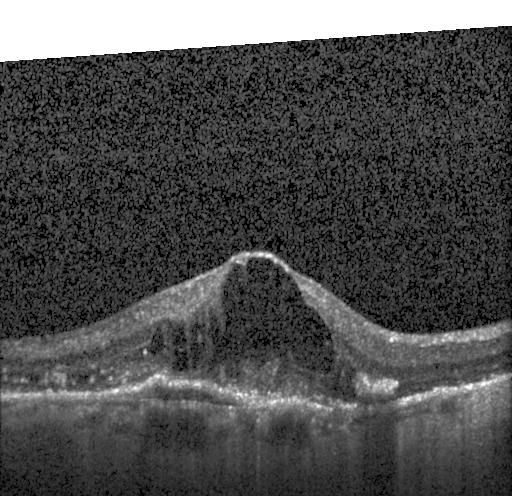

Retinal OCT cross-section, spectral-domain OCT
Finding: choroidal neovascularization (CNV).